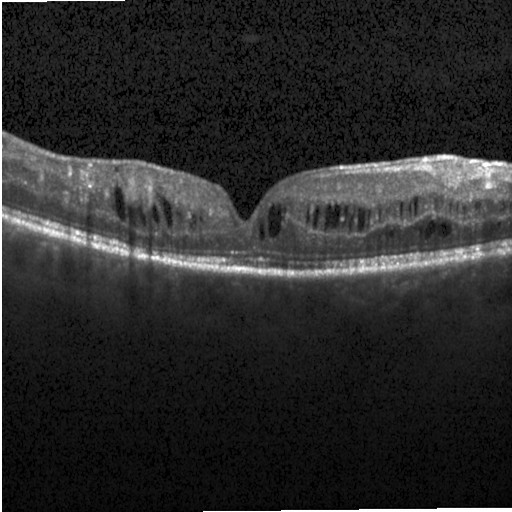 Macular scan; retinal OCT cross-section; instrument: Heidelberg Spectralis; spectral-domain optical coherence tomography
Macular OCT: diabetic macular edema.